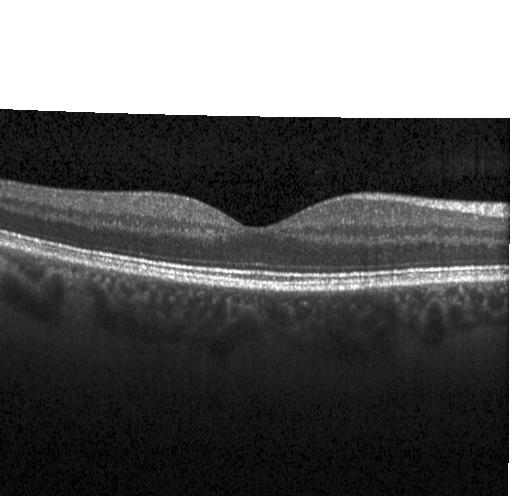
Macular OCT: no evidence of CNV, DME, or drusen.